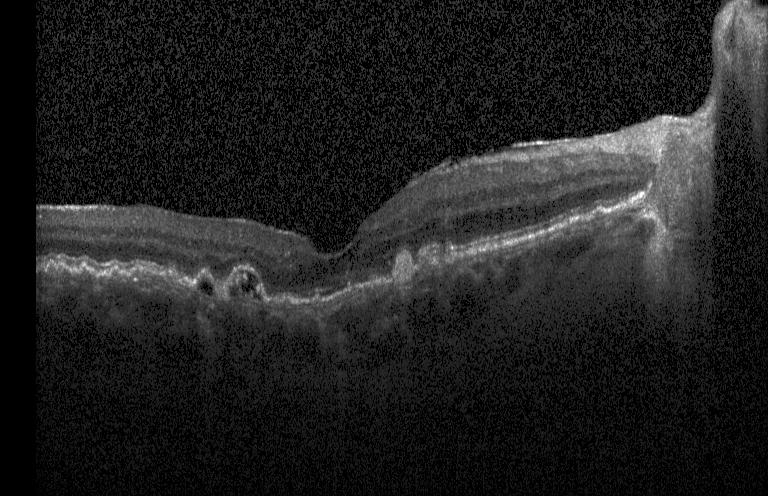

Fovea-centered. OCT B-scan. Acquired on a Heidelberg Spectralis. Spectral-domain optical coherence tomography — Assessment: choroidal neovascularization (CNV).